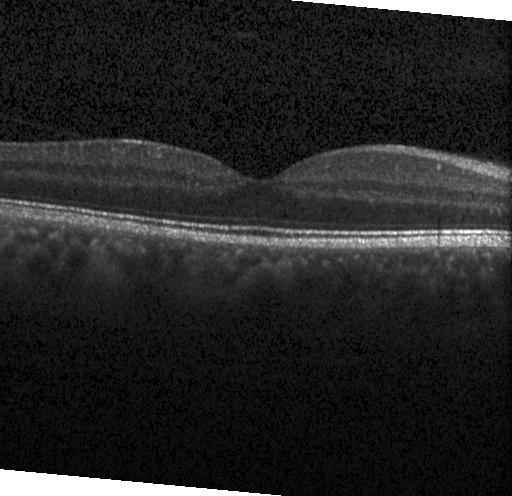 Through the macula · OCT B-scan — Dx: no choroidal neovascularization, diabetic macular edema, or drusen.